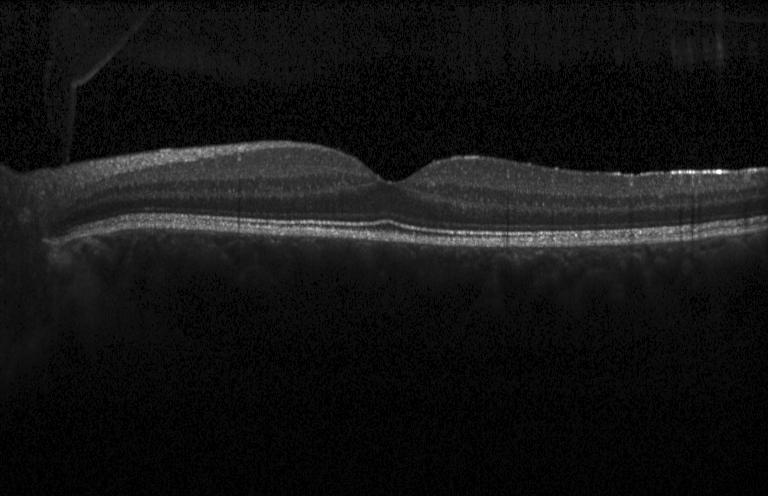 Dx: neither choroidal neovascularization, diabetic macular edema, nor drusen.